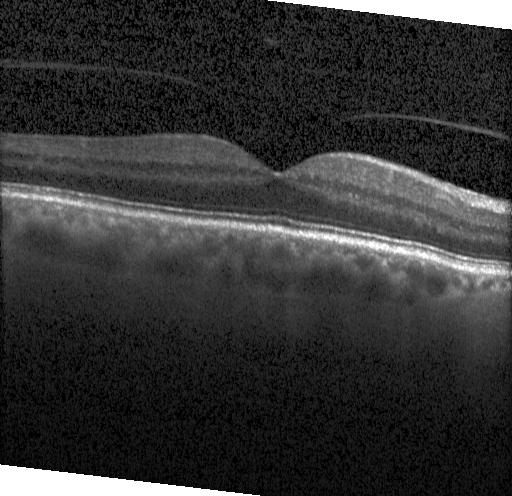 OCT line scan.
Diagnosis: neither choroidal neovascularization, diabetic macular edema, nor drusen.